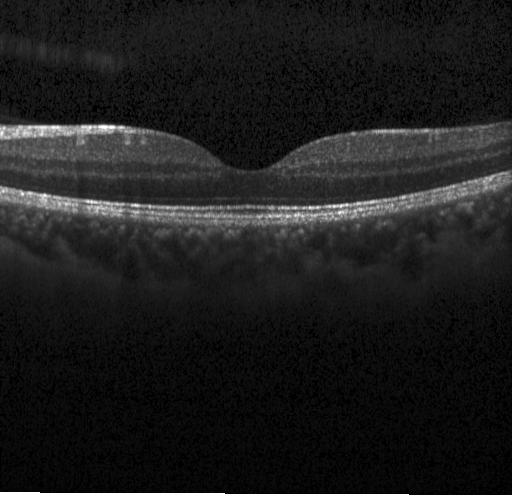 Retinal OCT cross-section.
This B-scan demonstrates no evidence of CNV, DME, or drusen.